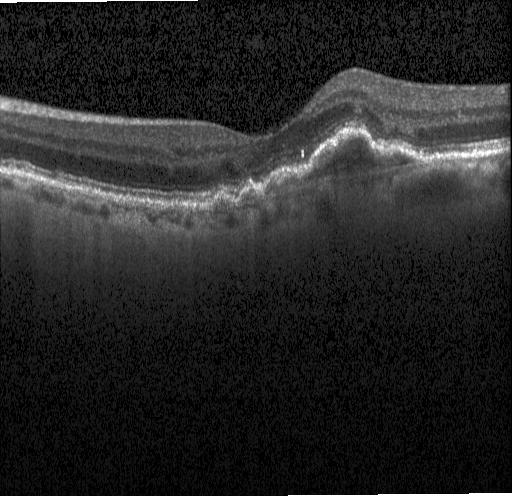 Macular OCT: choroidal neovascularization (CNV).